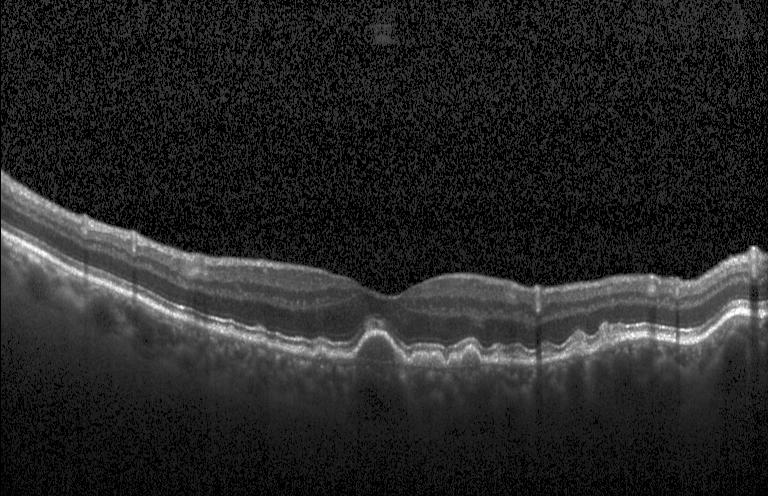 Drusen.